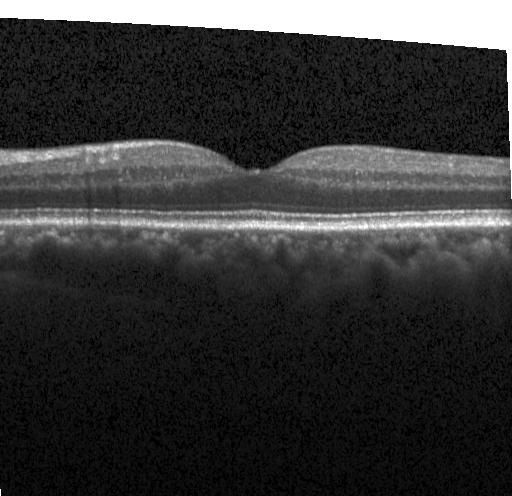 OCT line scan.
The scan shows no evidence of choroidal neovascularization, diabetic macular edema, or drusen.